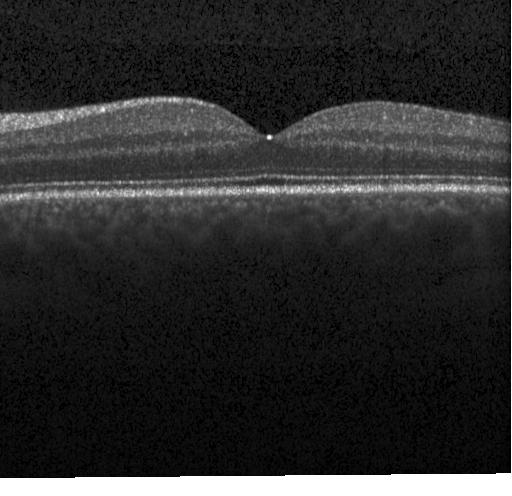

Finding: no CNV, no DME, and no drusen.